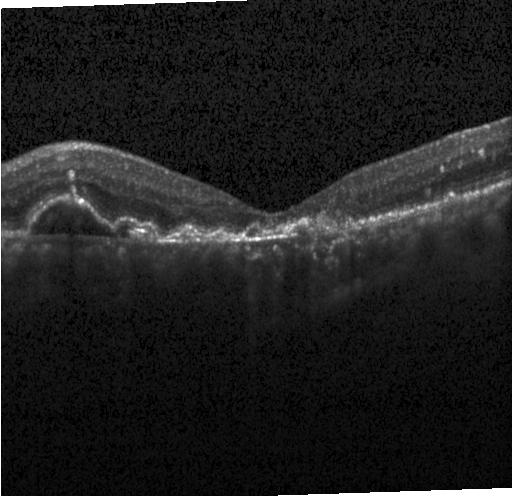
Spectral-domain OCT · acquired on a Heidelberg Spectralis · macular scan · OCT B-scan. Diagnosis: a choroidal neovascular membrane.